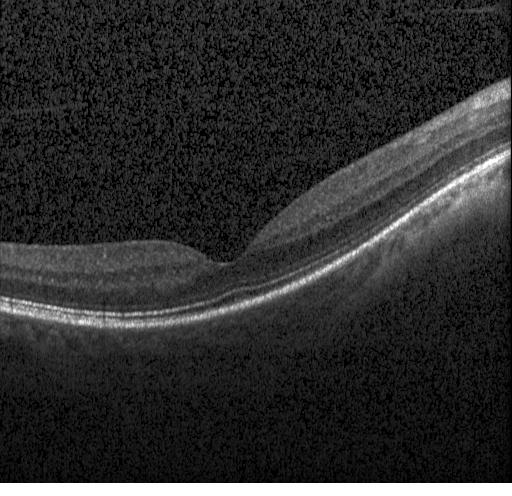

Spectral-domain OCT B-scan: neither choroidal neovascularization, diabetic macular edema, nor drusen.